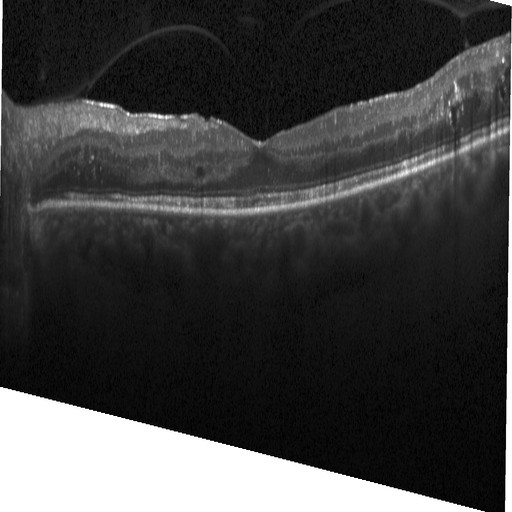 The scan shows DME.